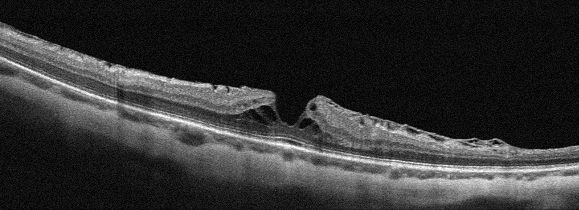

Oculus sinister, OCT line scan
VID.